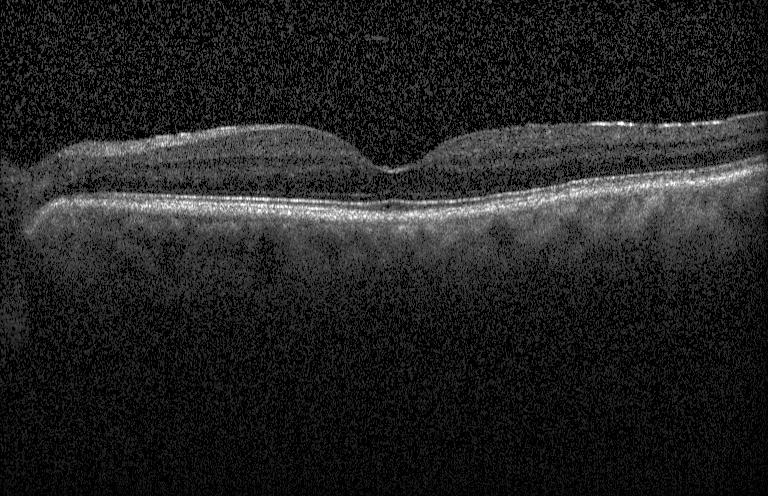
OCT line scan. Macular scan — This B-scan demonstrates no evidence of CNV, DME, or drusen.